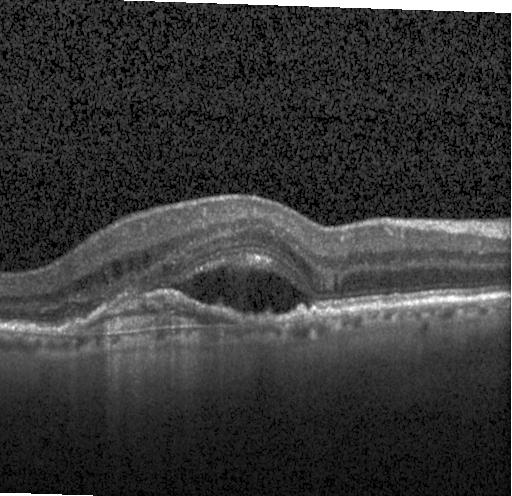 OCT line scan. Impression: a choroidal neovascular membrane.